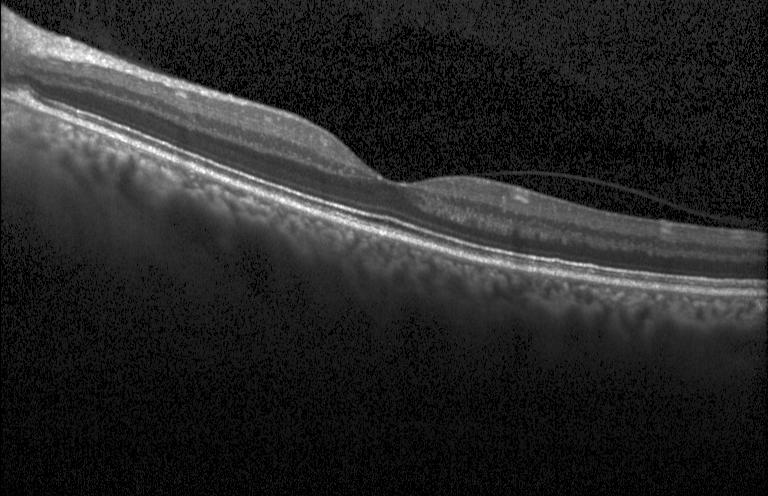

OCT B-scan · SD-OCT. Assessment: no evidence of CNV, DME, or drusen.